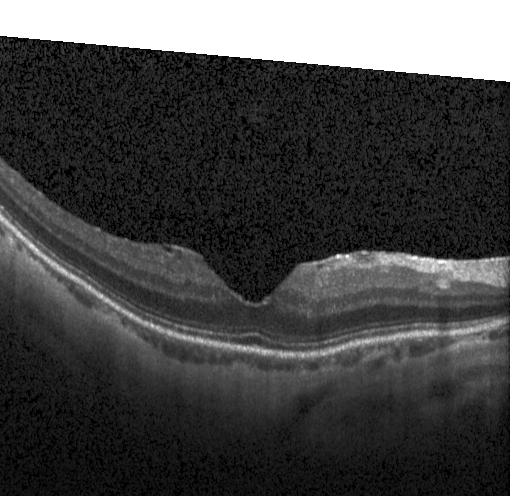 The scan shows no CNV, no DME, and no drusen.